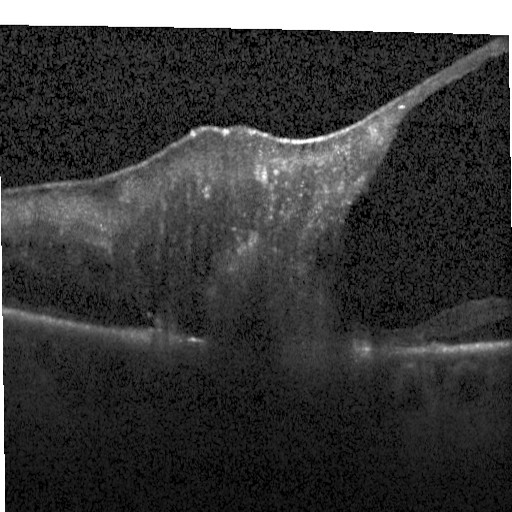

Retinal OCT cross-section; macular scan; SD-OCT.
Diabetic macular edema (DME).